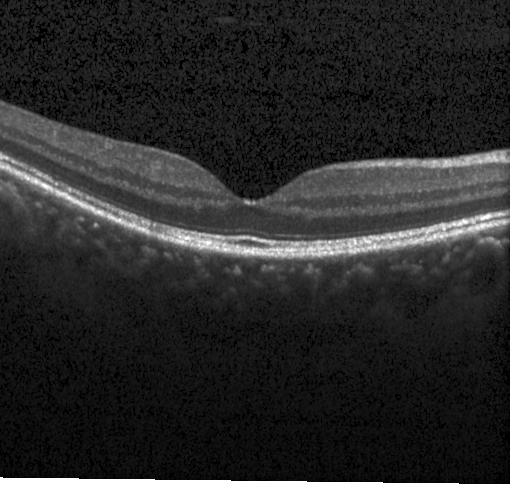
SD-OCT; macular scan; OCT B-scan — This B-scan demonstrates no choroidal neovascularization, diabetic macular edema, or drusen.